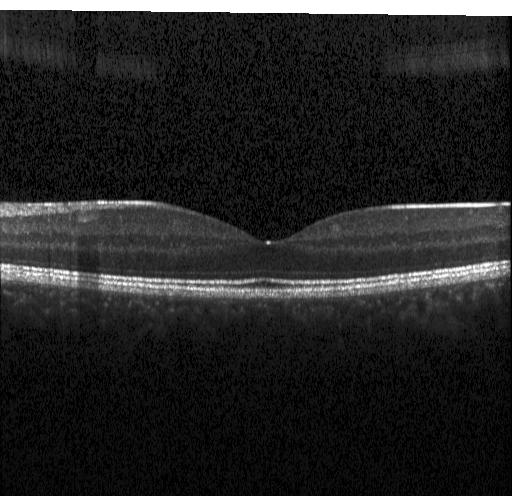
Optical coherence tomography B-scan. Through the macula. Heidelberg Spectralis. Spectral-domain OCT — Finding: no CNV, no DME, and no drusen.